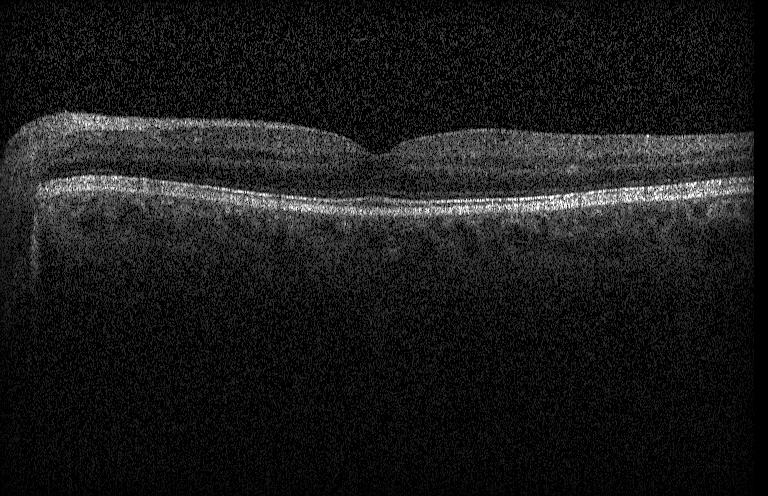 This B-scan demonstrates no CNV, DME, or drusen.